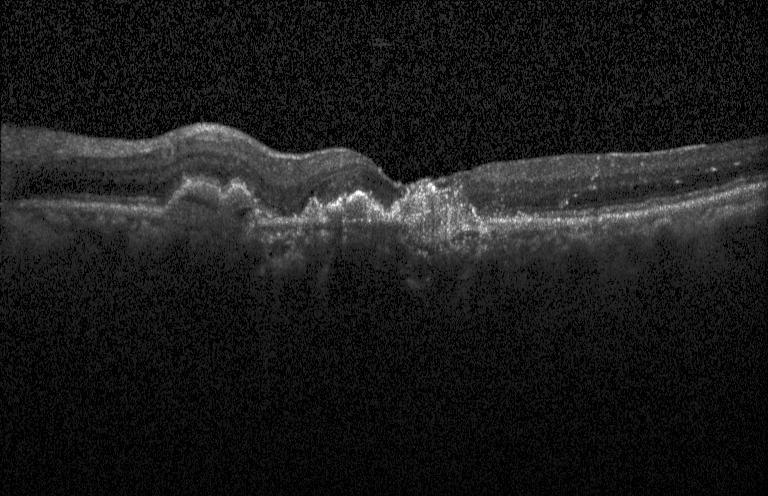 OCT finding: choroidal neovascularization (CNV).